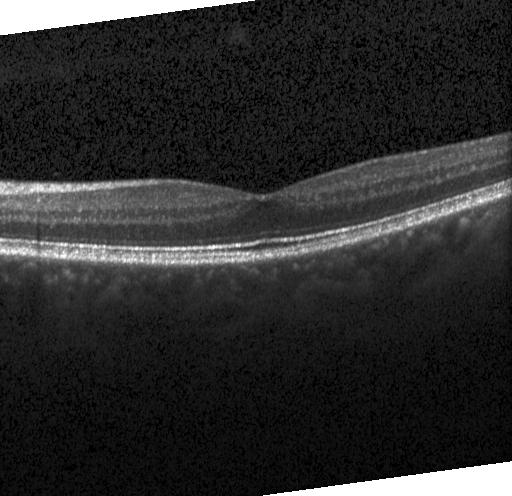

Retinal OCT B-scan; fovea-centered
Diagnosis: no choroidal neovascularization, diabetic macular edema, or drusen.